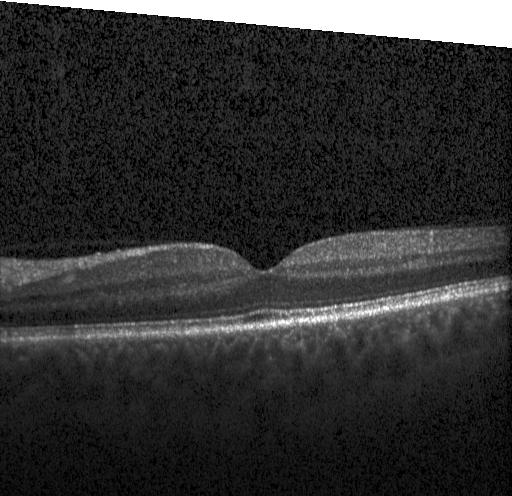 Impression: no CNV, DME, or drusen.